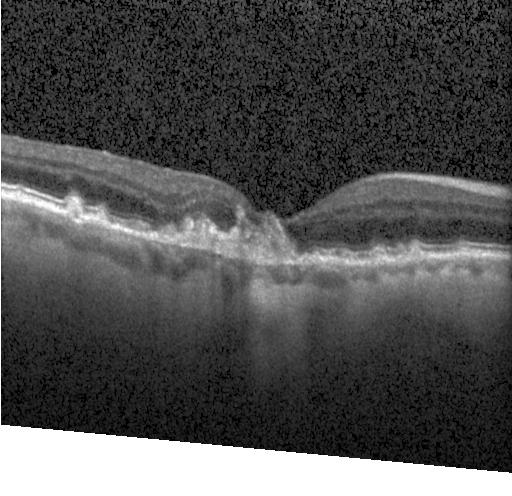 Heidelberg Spectralis OCT system, retinal OCT B-scan, through the macula, spectral-domain OCT. A choroidal neovascular membrane.